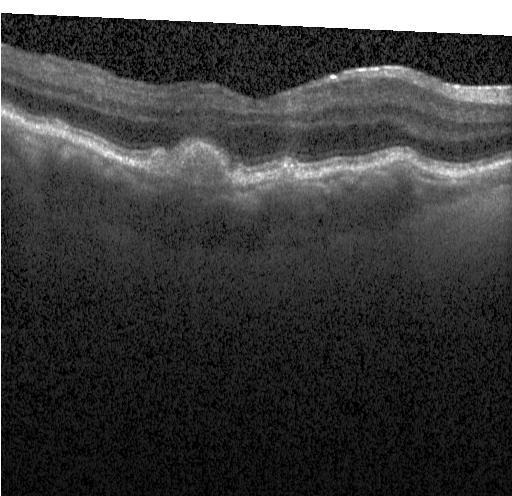
OCT line scan. Centered on the fovea. Heidelberg Spectralis. Spectral-domain OCT
Diagnosis: choroidal neovascularization (CNV).